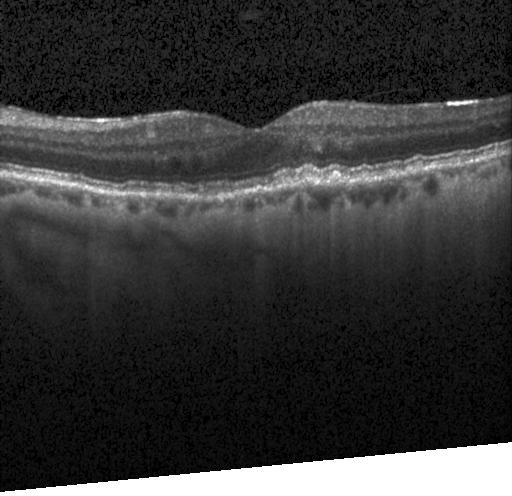 OCT scan showing multiple drusen.